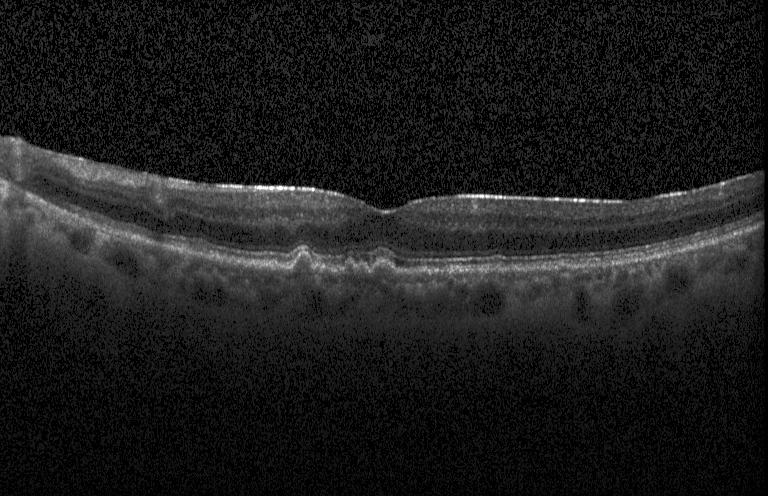
Optical coherence tomography B-scan. This B-scan demonstrates multiple drusen.